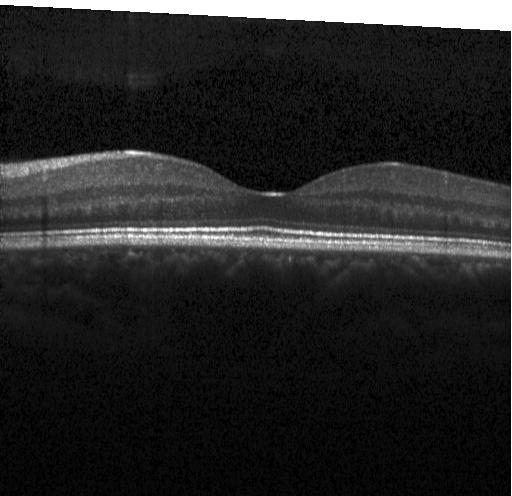 Retinal OCT B-scan
OCT finding: no evidence of choroidal neovascularization, diabetic macular edema, or drusen.